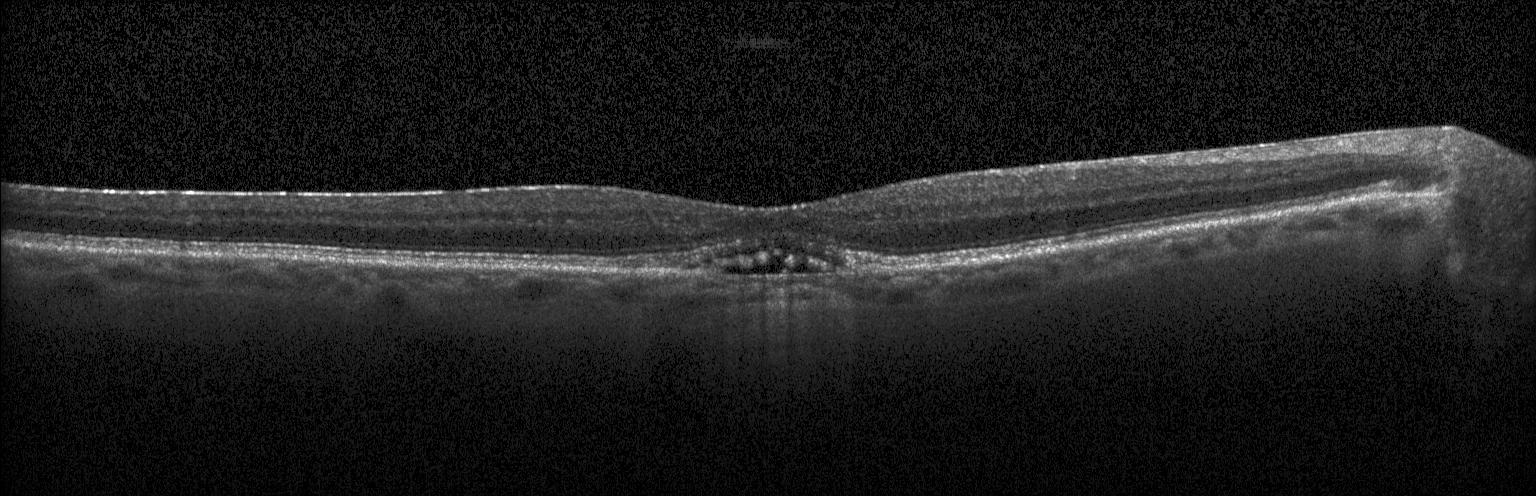 Macular scan, optical coherence tomography scan, Heidelberg Spectralis. The scan shows a choroidal neovascular membrane.